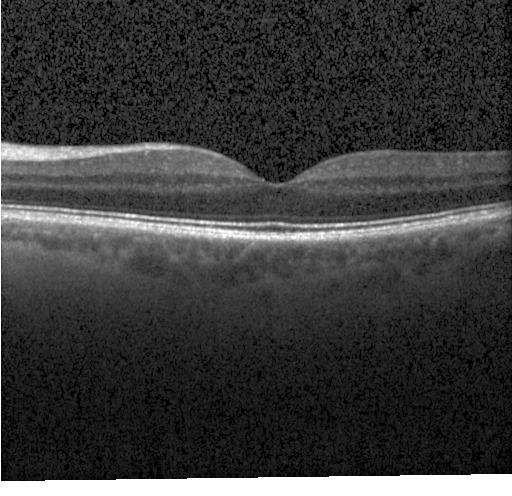
Diagnosis: neither choroidal neovascularization, diabetic macular edema, nor drusen.